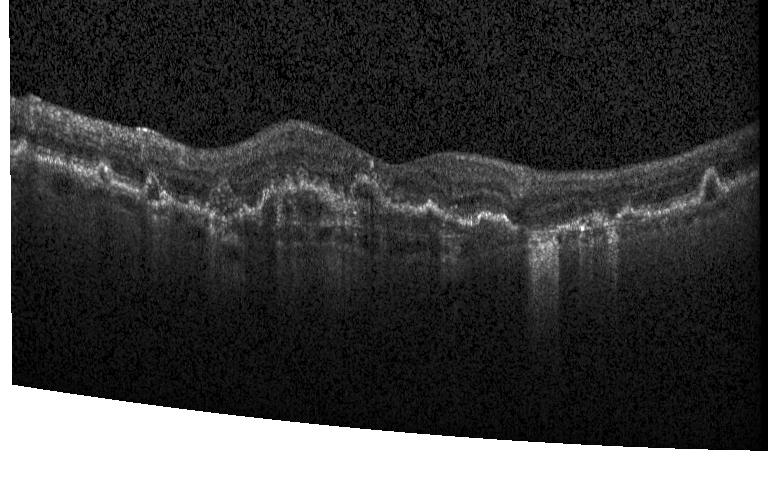

Heidelberg Spectralis, retinal OCT cross-section, SD-OCT
The scan shows CNV.